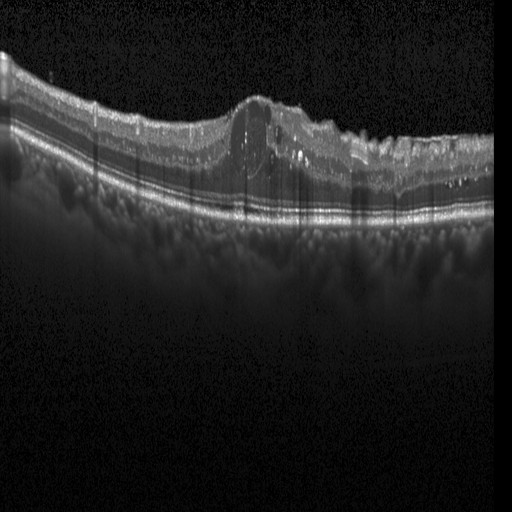

OCT line scan, through the macula — This B-scan demonstrates diabetic macular edema (DME).